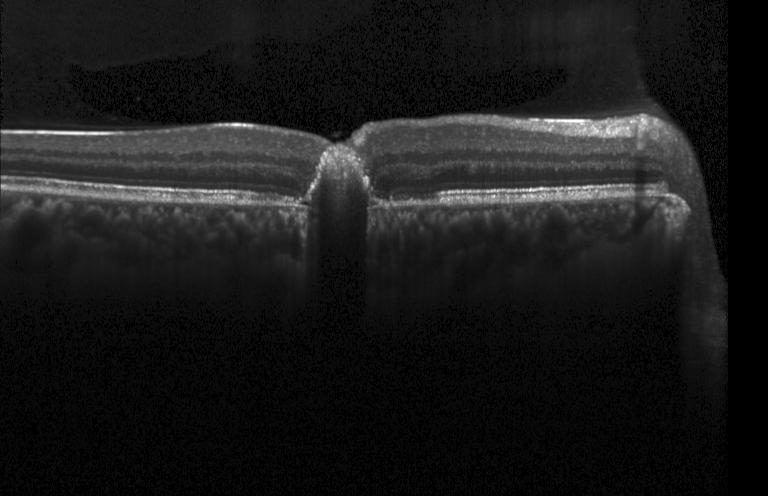 The scan shows a choroidal neovascular membrane.